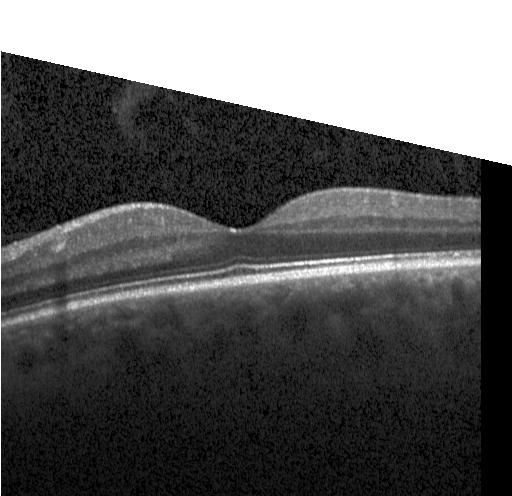 Impression: neither choroidal neovascularization, diabetic macular edema, nor drusen.